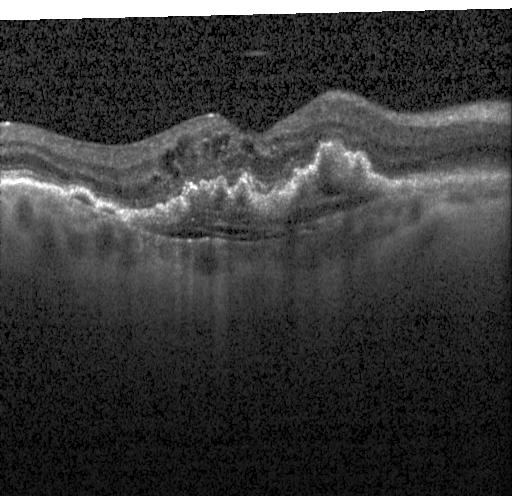 Through the macula · OCT B-scan · acquired on a Heidelberg Spectralis
Diagnosis: a choroidal neovascular membrane.